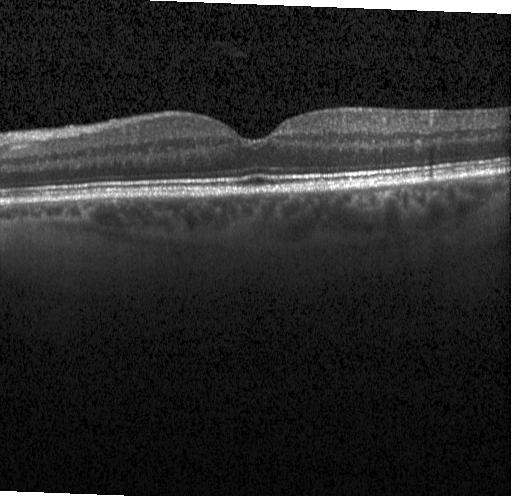

OCT finding: no choroidal neovascularization, no diabetic macular edema, and no drusen.